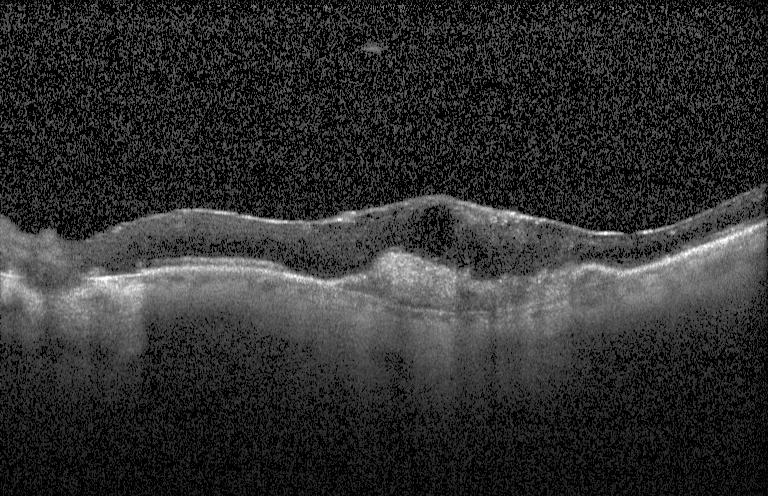 Optical coherence tomography scan · SD-OCT
Assessment: CNV.